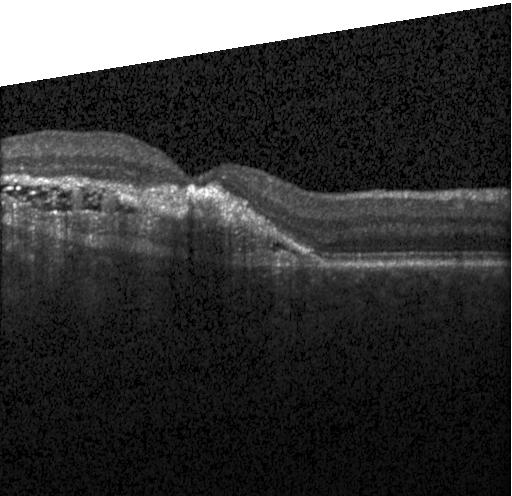

Fovea-centered. Acquired on a Heidelberg Spectralis. Optical coherence tomography B-scan
Impression: choroidal neovascularization.